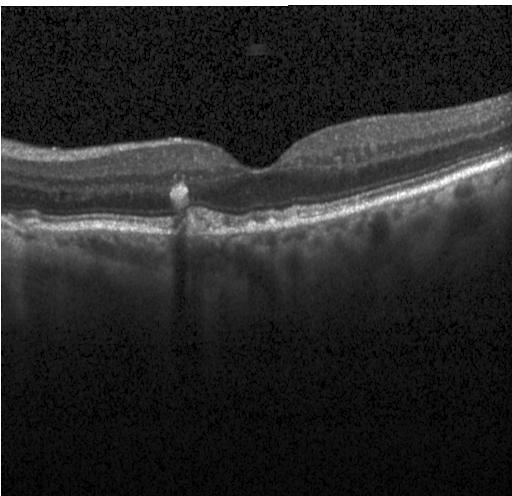 Heidelberg Spectralis, SD-OCT, retinal OCT B-scan.
This B-scan demonstrates drusen.